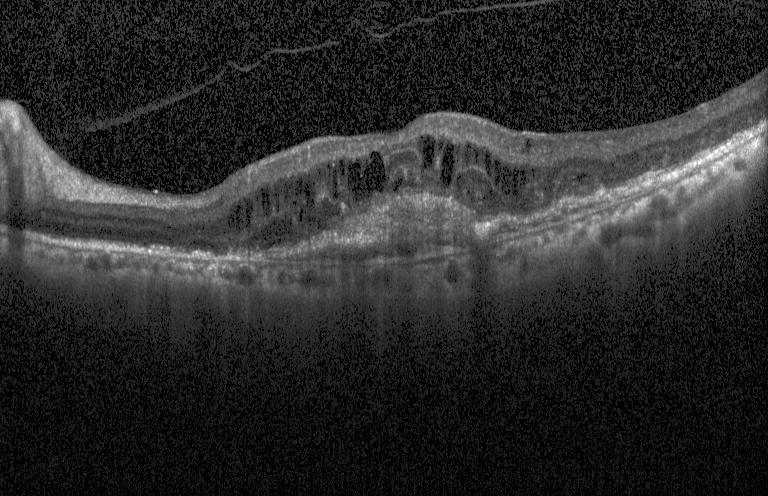 Macular OCT demonstrating a choroidal neovascular membrane.